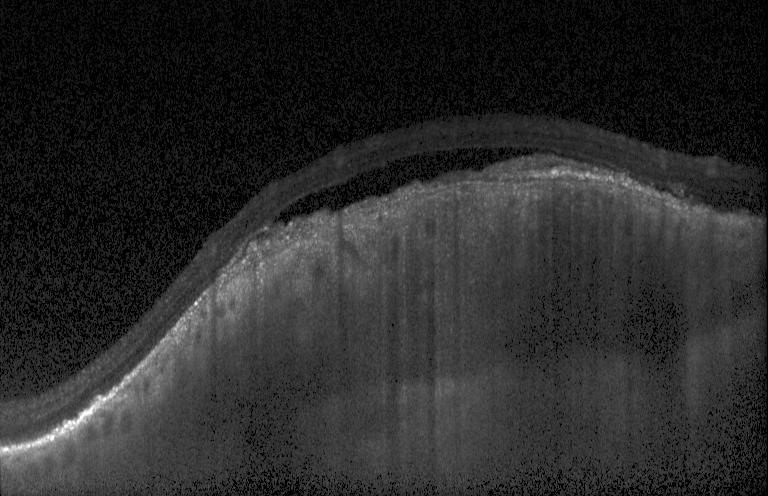
Retinal OCT B-scan, Heidelberg Spectralis, spectral-domain optical coherence tomography.
This B-scan demonstrates a choroidal neovascular membrane.